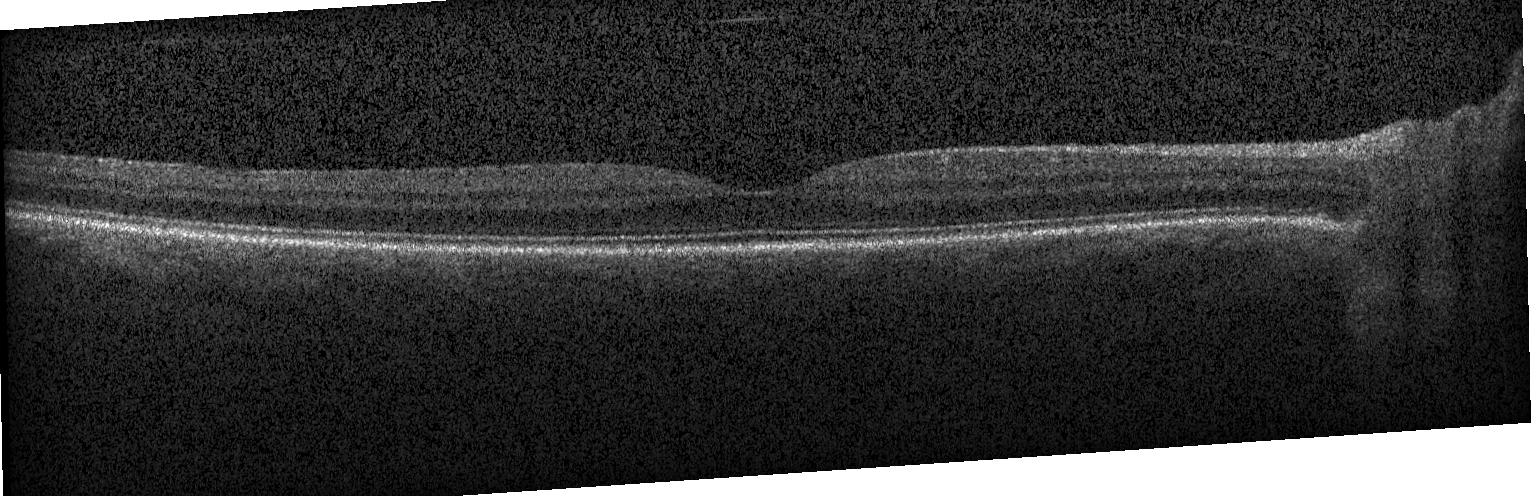
Retinal OCT B-scan · SD-OCT · centered on the fovea
Impression: no CNV, no DME, and no drusen.